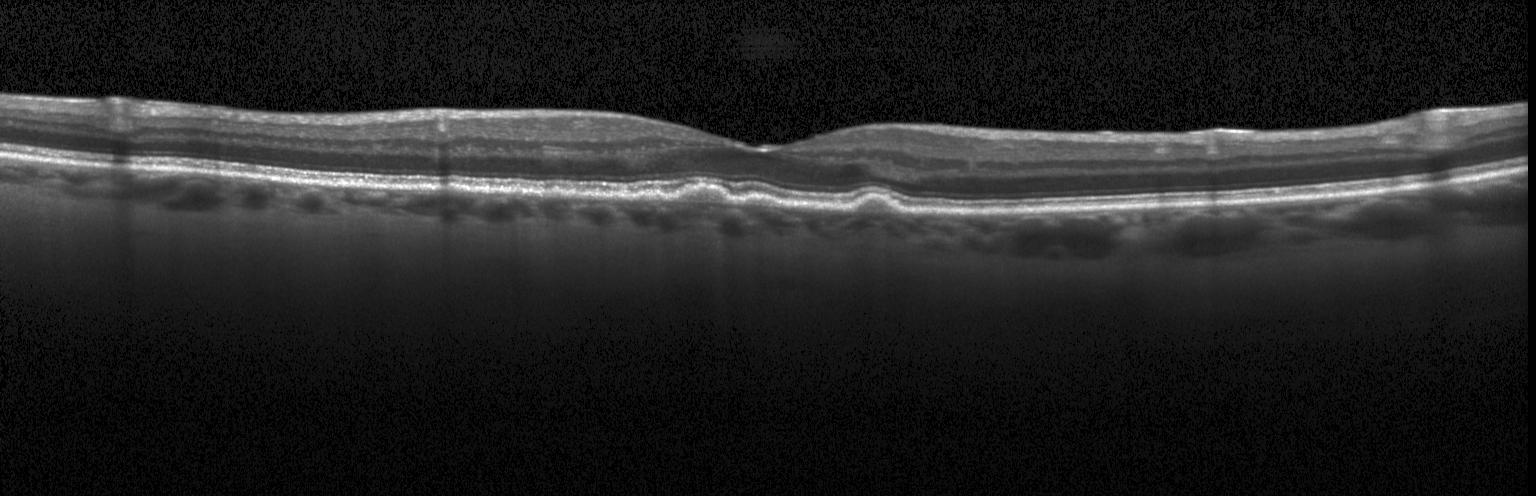
OCT finding: sub-RPE drusenoid deposits.